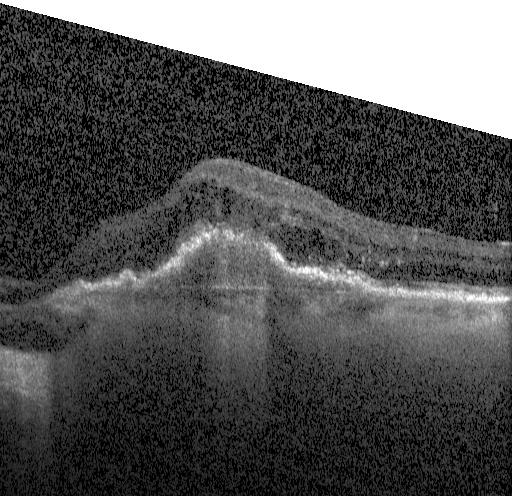

Retinal OCT cross-section, fovea-centered, spectral-domain OCT — Finding: choroidal neovascularization.